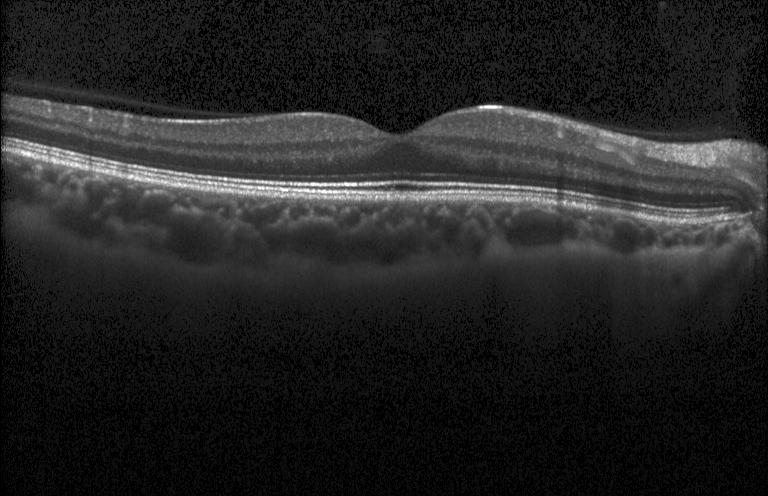
Retinal OCT B-scan, spectral-domain optical coherence tomography, instrument: Heidelberg Spectralis
Assessment: no choroidal neovascularization, diabetic macular edema, or drusen.